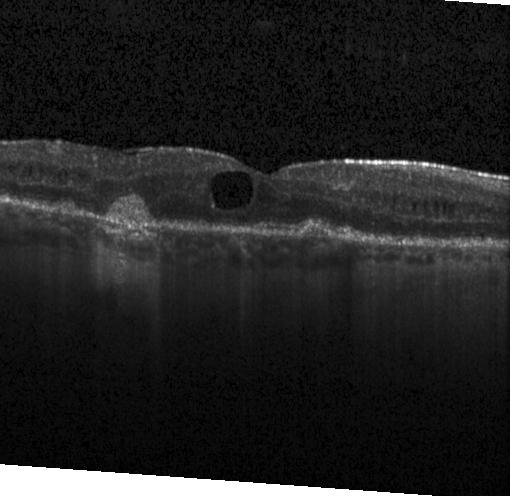 OCT B-scan; through the macula.
Diagnosis: choroidal neovascularization.